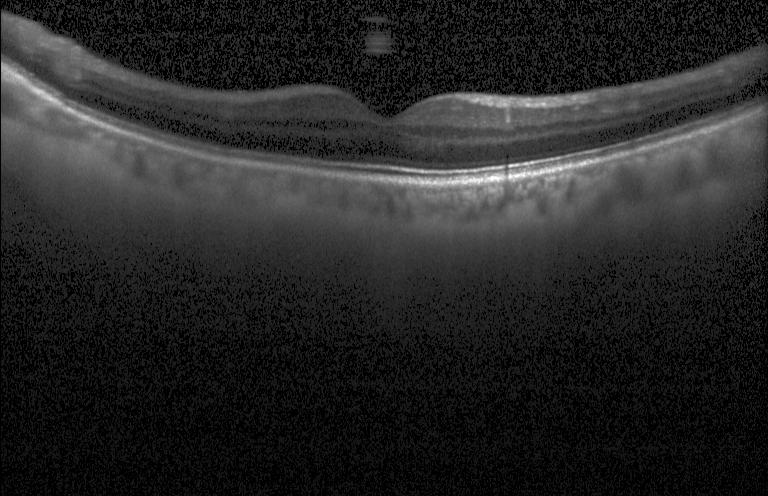
Acquired on a Heidelberg Spectralis · spectral-domain OCT · retinal OCT B-scan · macular scan — OCT finding: neither choroidal neovascularization, diabetic macular edema, nor drusen.